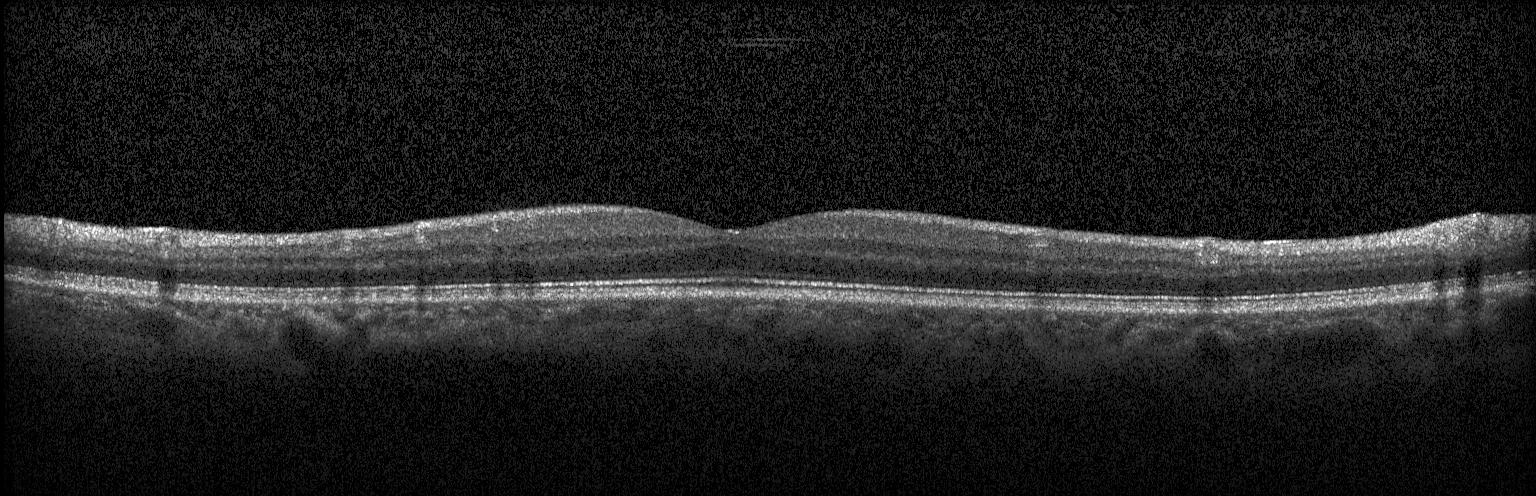

OCT line scan — Finding: neither choroidal neovascularization, diabetic macular edema, nor drusen.